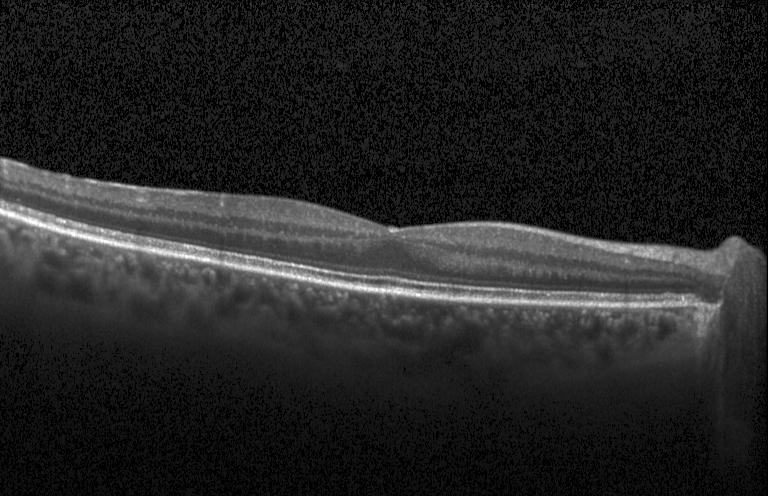 Finding: no CNV, DME, or drusen.